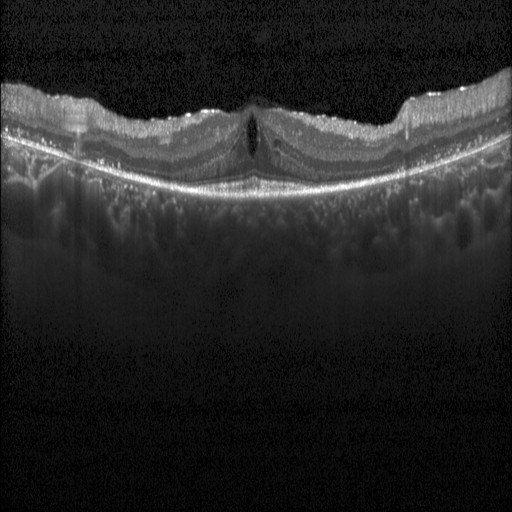
SD-OCT; instrument: Heidelberg Spectralis; horizontal scan through the fovea; OCT line scan
Dx: diabetic macular edema.